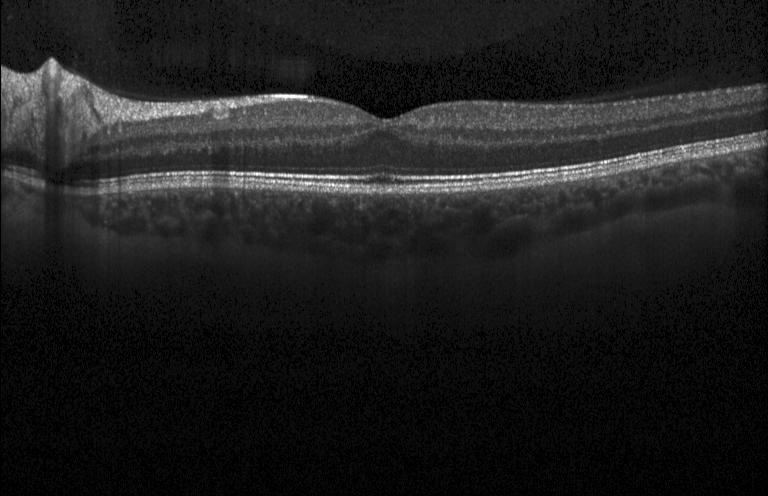 SD-OCT, horizontal scan through the fovea, OCT B-scan. The scan shows no choroidal neovascularization, diabetic macular edema, or drusen.